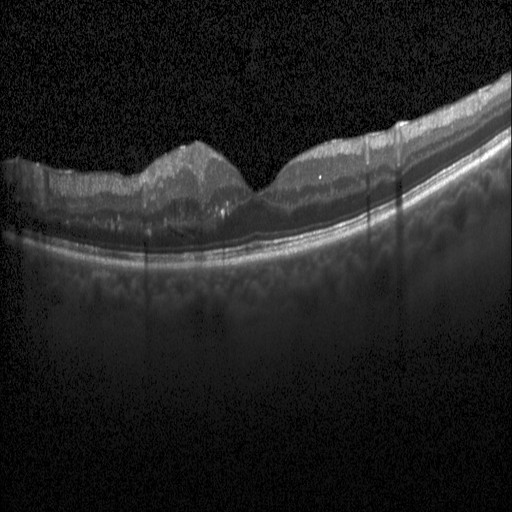 Centered on the fovea, retinal OCT cross-section, acquired on a Heidelberg Spectralis
Impression: diabetic macular edema (DME).